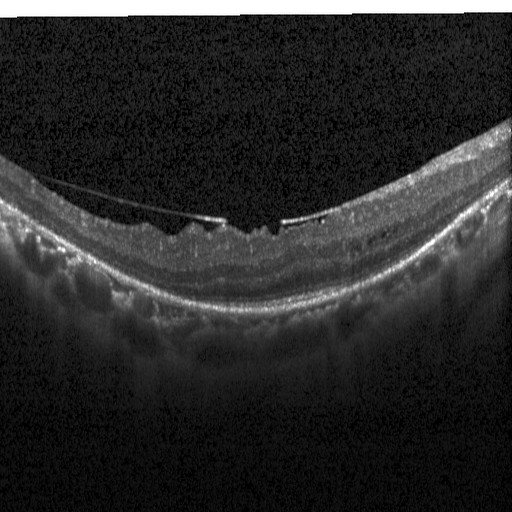

Retinal OCT B-scan
Diagnosis: diabetic macular edema (DME).